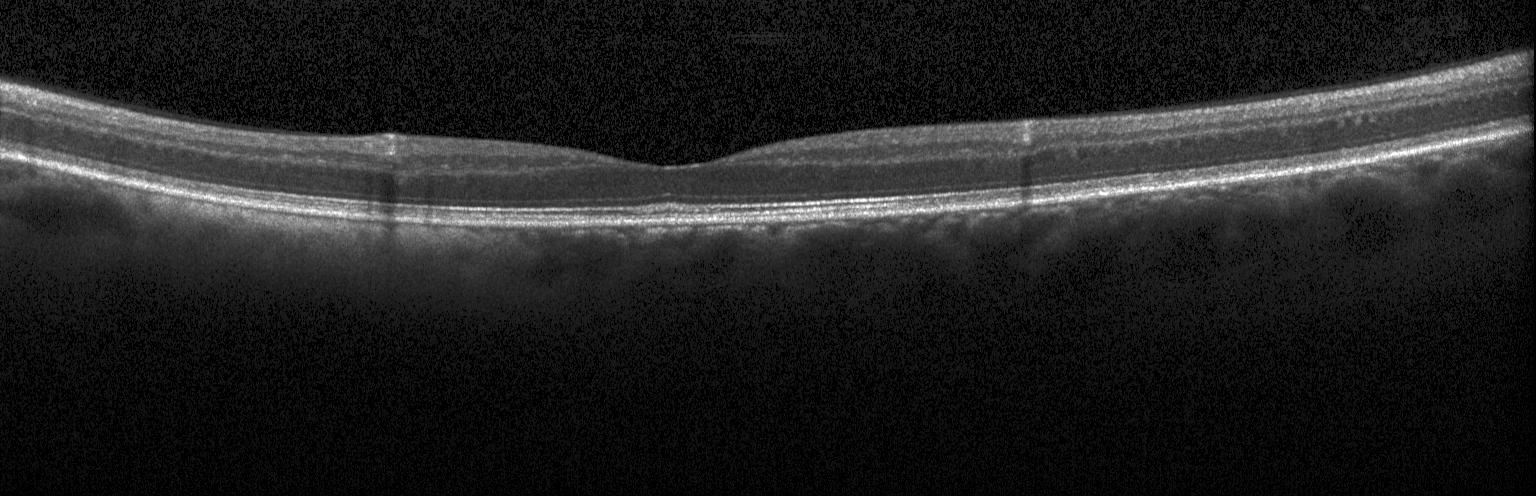 Heidelberg Spectralis; SD-OCT; OCT line scan; through the macula. Finding: neither choroidal neovascularization, diabetic macular edema, nor drusen.